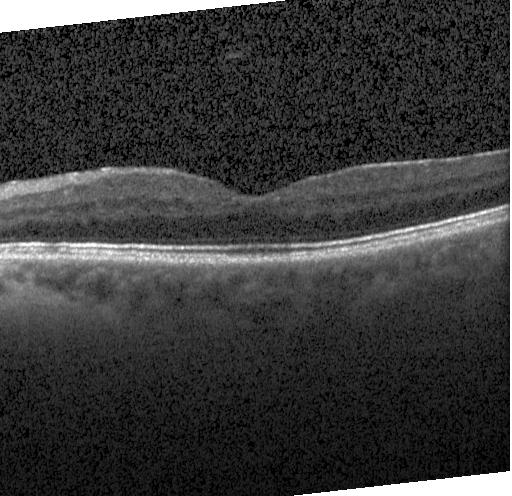
The scan shows neither choroidal neovascularization, diabetic macular edema, nor drusen.